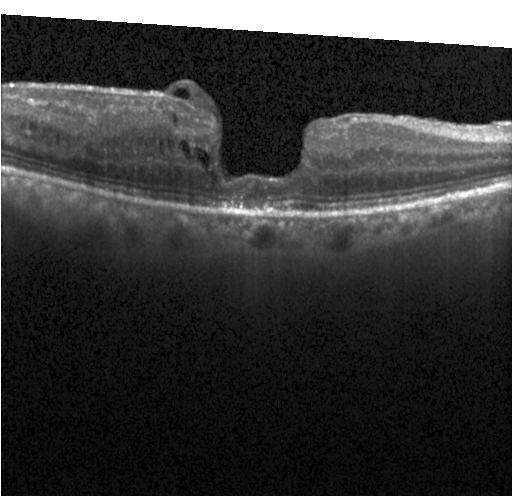

Macular OCT demonstrating DME.